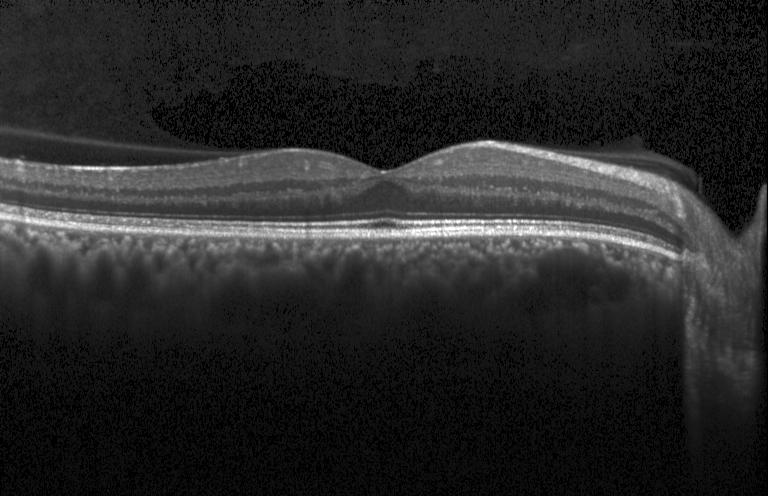
Retinal OCT cross-section showing no evidence of choroidal neovascularization, diabetic macular edema, or drusen.